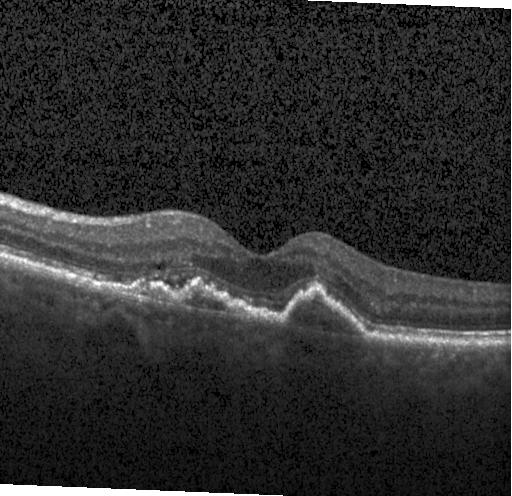

Retinal OCT B-scan · instrument: Heidelberg Spectralis · SD-OCT
Diagnosis: CNV.